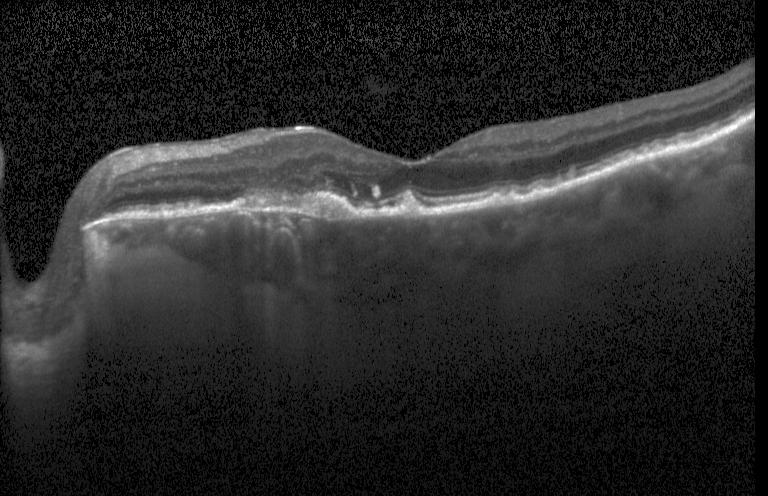

Finding: CNV.